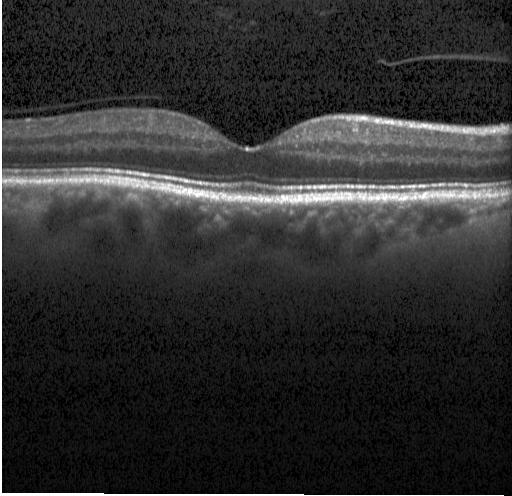

Diagnosis: no choroidal neovascularization, diabetic macular edema, or drusen.